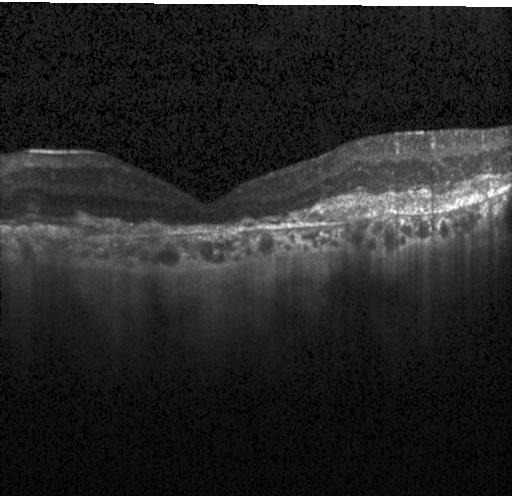
Horizontal scan through the fovea, spectral-domain optical coherence tomography, OCT B-scan, Heidelberg Spectralis
Impression: a choroidal neovascular membrane.